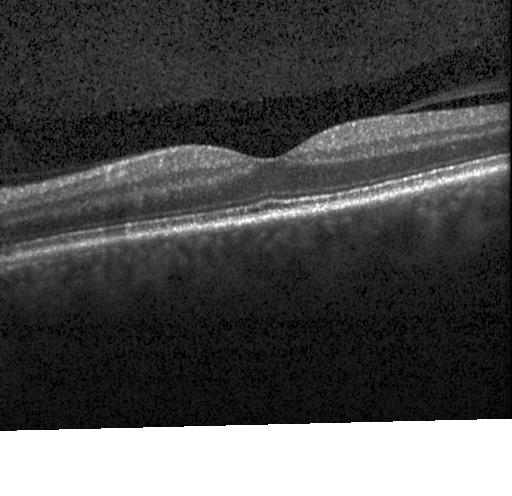

Assessment: no choroidal neovascularization, diabetic macular edema, or drusen.